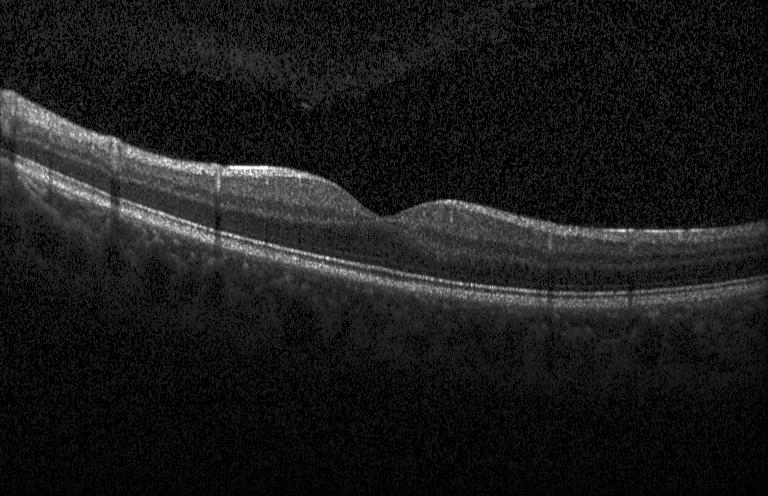
Finding: neither CNV, DME, nor drusen.